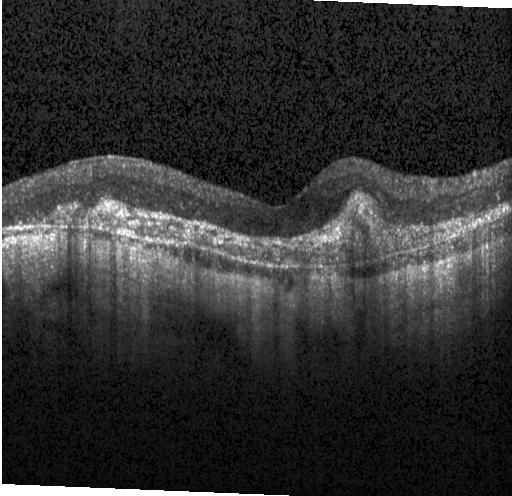 Retinal OCT cross-section.
Macular OCT: choroidal neovascularization.